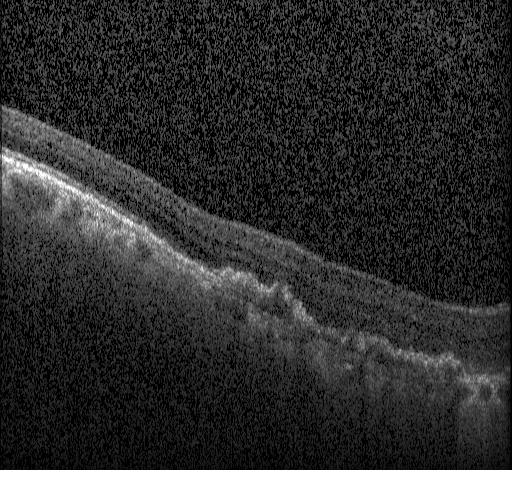

Through the macula · OCT B-scan · spectral-domain OCT · Heidelberg Spectralis — This B-scan demonstrates CNV.